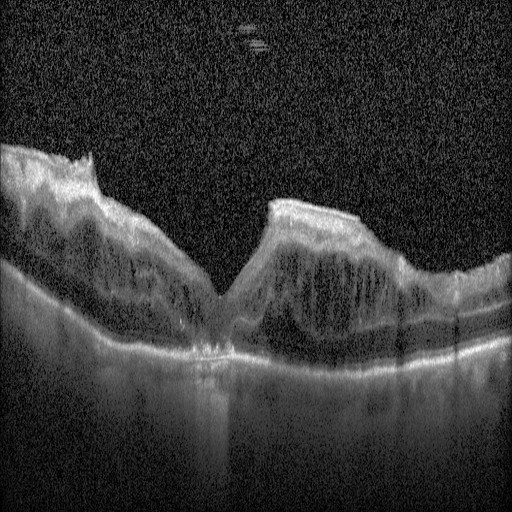

Heidelberg Spectralis; spectral-domain optical coherence tomography; optical coherence tomography B-scan. Diagnosis: diabetic macular edema.